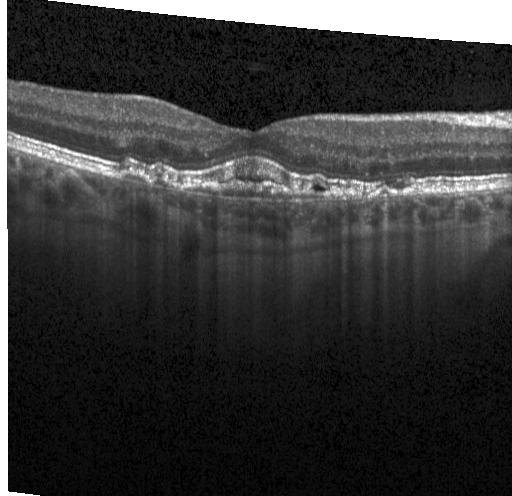 Through the macula · instrument: Heidelberg Spectralis · OCT line scan — CNV.